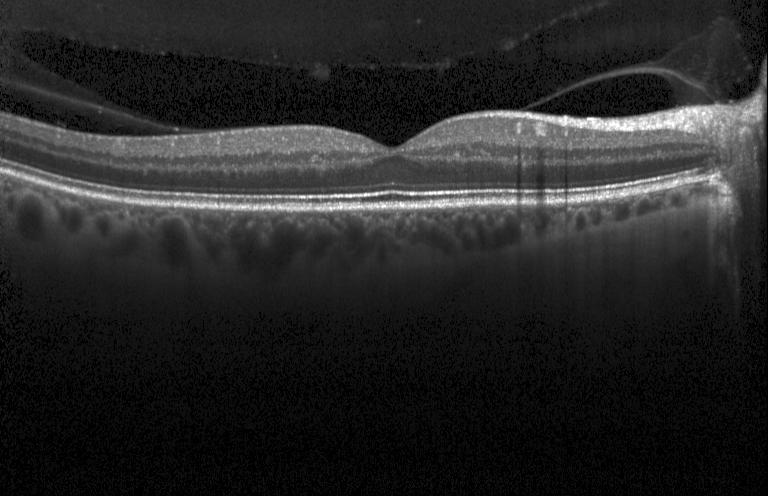
Macular scan; retinal OCT B-scan — Macular OCT: neither CNV, DME, nor drusen.